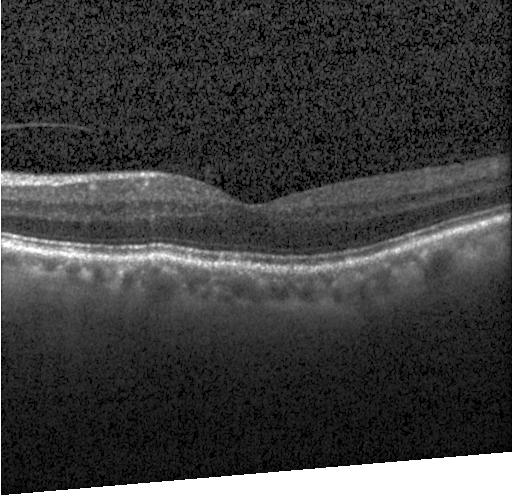 Heidelberg Spectralis OCT system, macular scan, optical coherence tomography B-scan, spectral-domain OCT
Impression: no choroidal neovascularization, diabetic macular edema, or drusen.